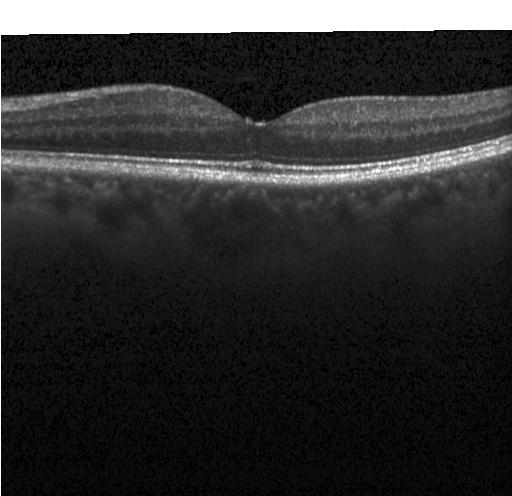
Fovea-centered, optical coherence tomography scan.
Finding: no CNV, DME, or drusen.